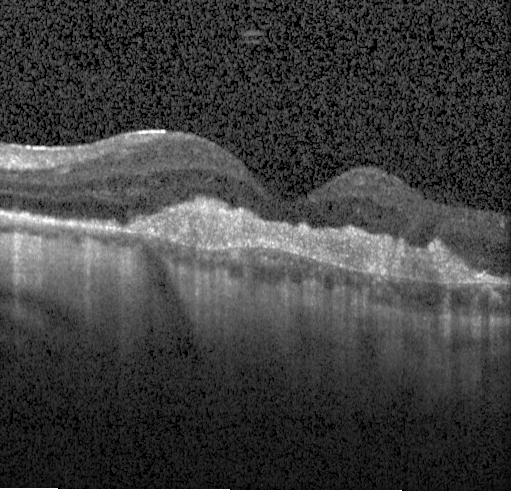

Acquired on a Heidelberg Spectralis, optical coherence tomography scan.
Dx: choroidal neovascularization (CNV).